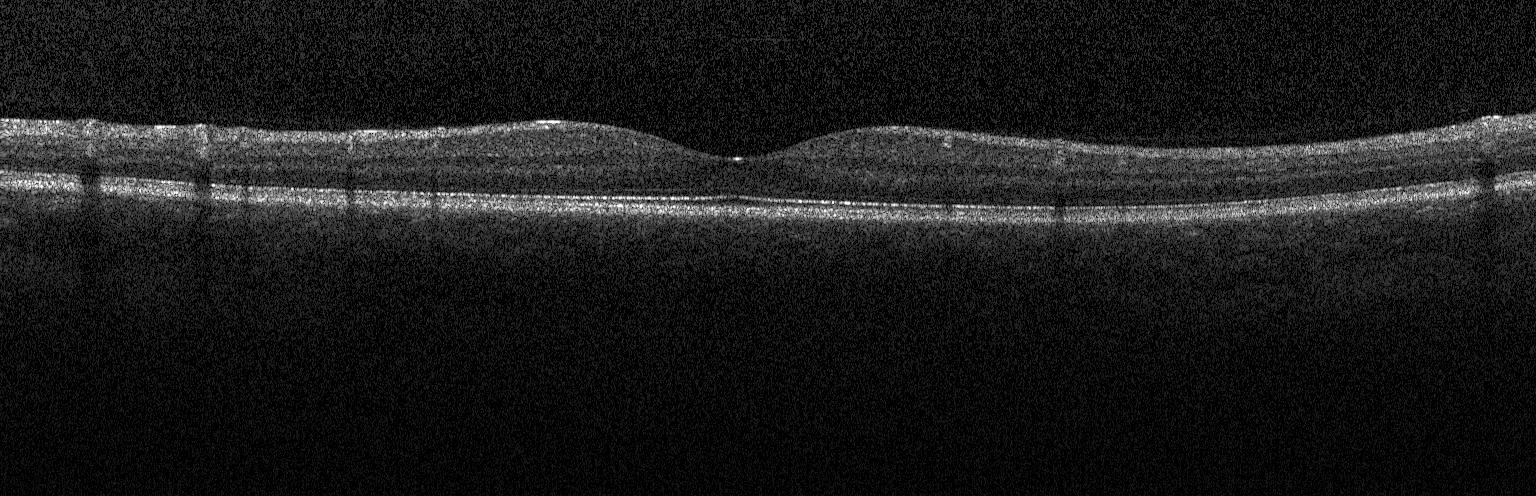 No CNV, no DME, and no drusen.